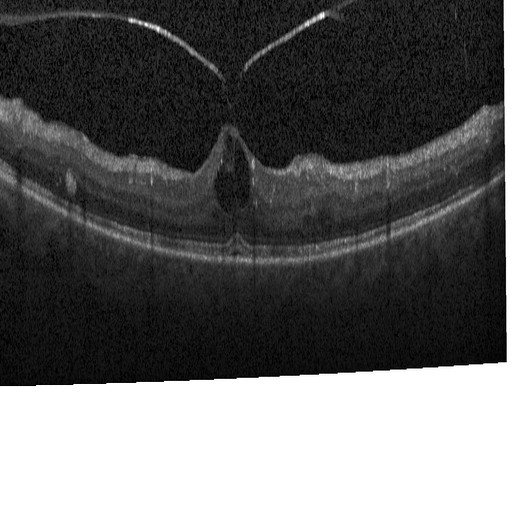

OCT B-scan — Assessment: DME.